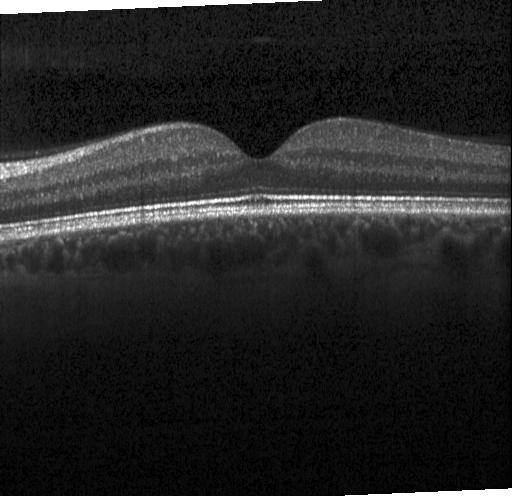

Impression: no evidence of choroidal neovascularization, diabetic macular edema, or drusen.